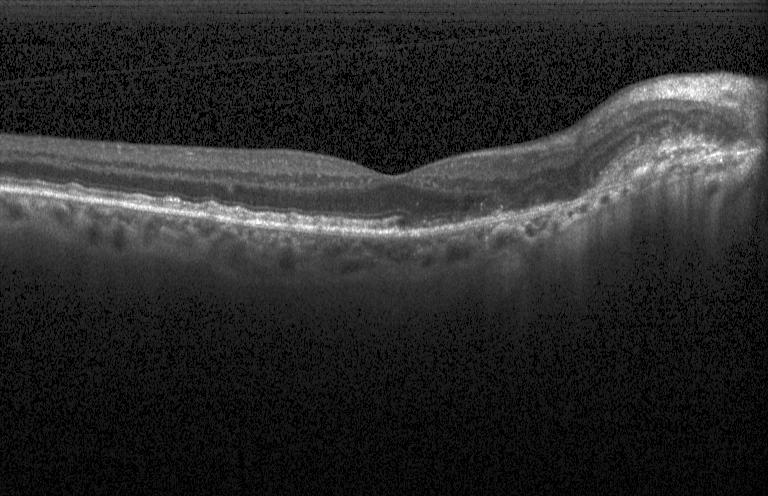
Spectral-domain OCT B-scan: CNV.